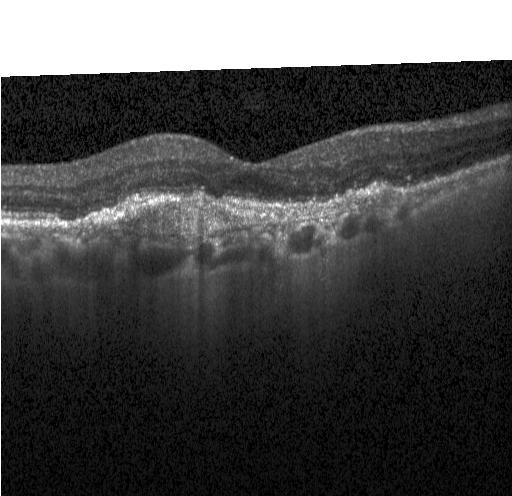 Diagnosis: a choroidal neovascular membrane.